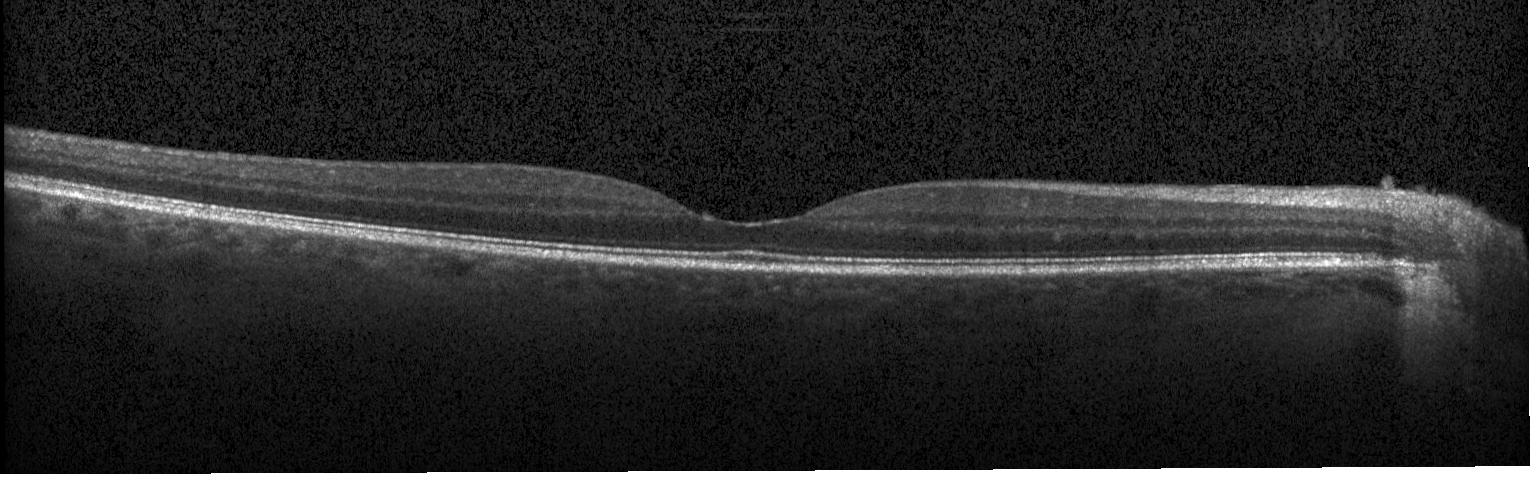

Spectral-domain optical coherence tomography; macular scan; optical coherence tomography scan; instrument: Heidelberg Spectralis — This B-scan demonstrates neither choroidal neovascularization, diabetic macular edema, nor drusen.